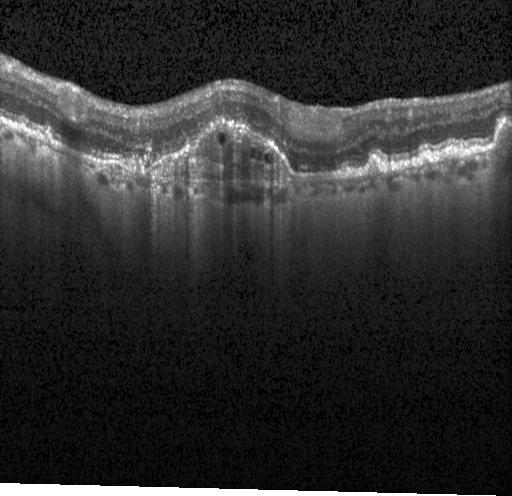

OCT B-scan · spectral-domain OCT — Impression: choroidal neovascularization (CNV).